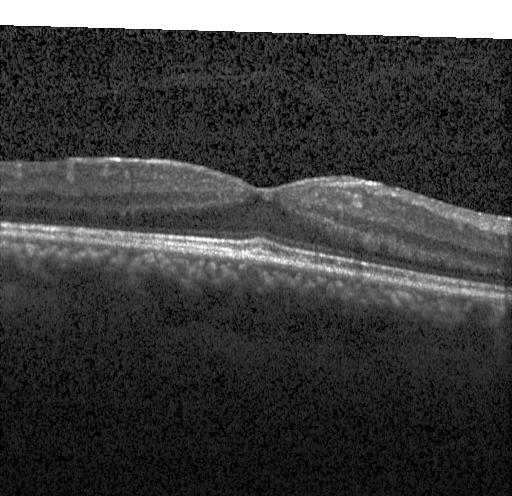

OCT B-scan — No evidence of choroidal neovascularization, diabetic macular edema, or drusen.